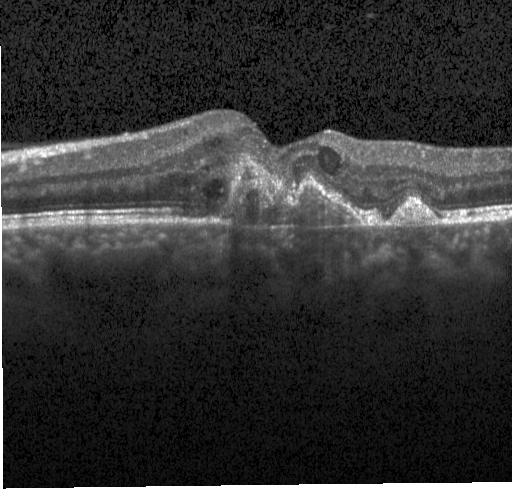 Retinal OCT cross-section · through the macula · Heidelberg Spectralis.
OCT finding: CNV.